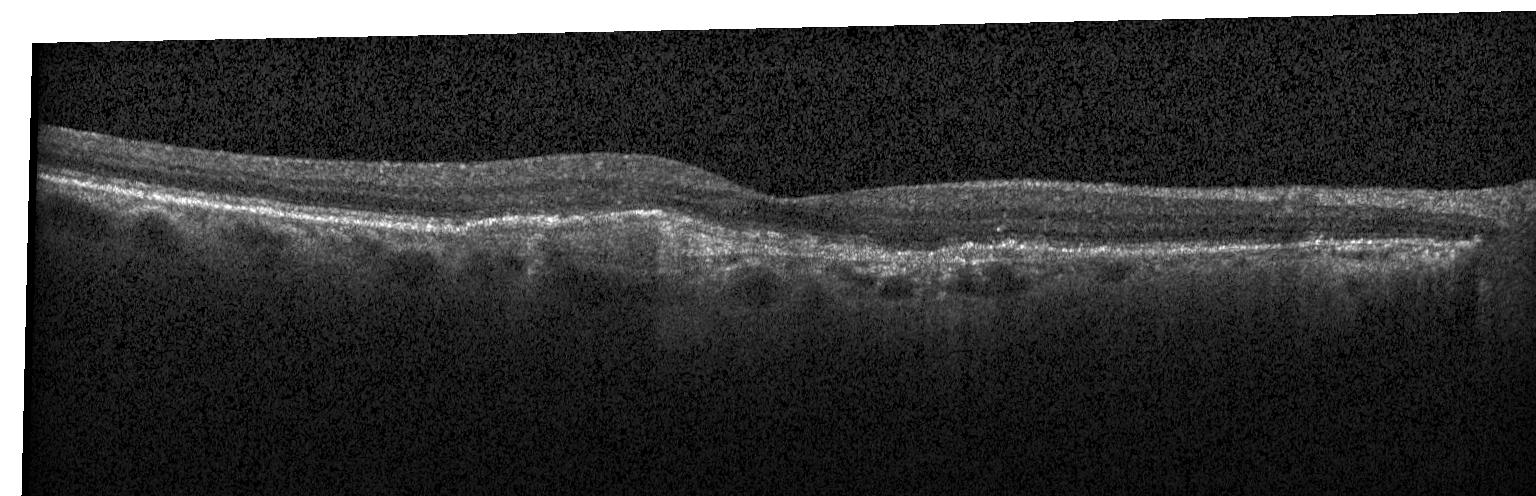
Macular OCT: a choroidal neovascular membrane.